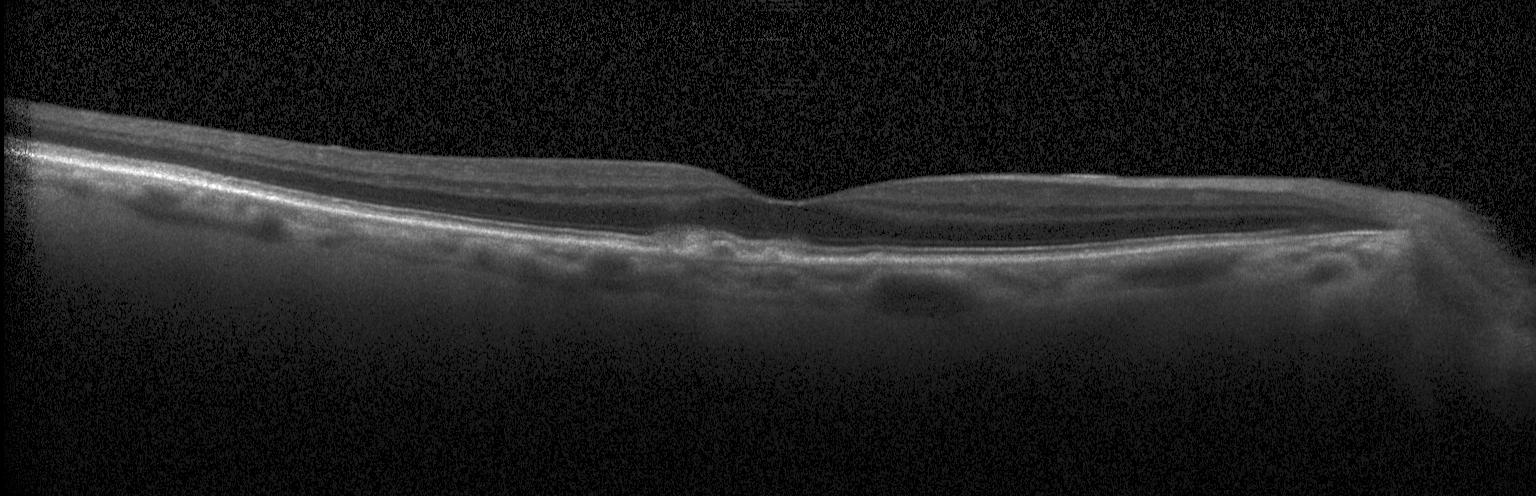

OCT scan showing multiple drusen.